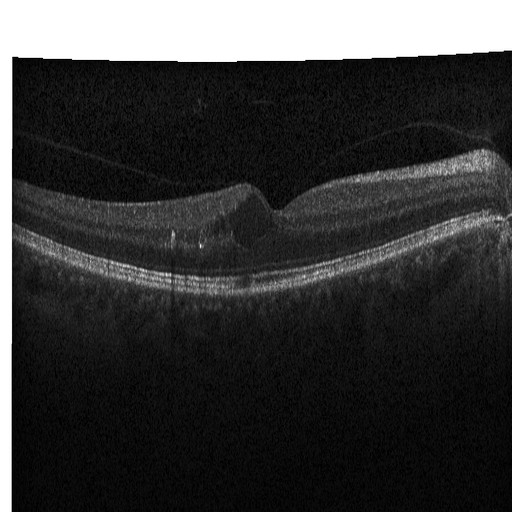
Retinal OCT cross-section showing DME.